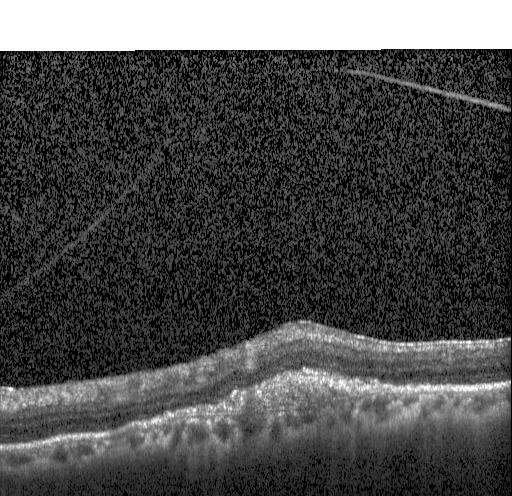

Heidelberg Spectralis OCT system; fovea-centered; SD-OCT; OCT line scan — Macular OCT: a choroidal neovascular membrane.